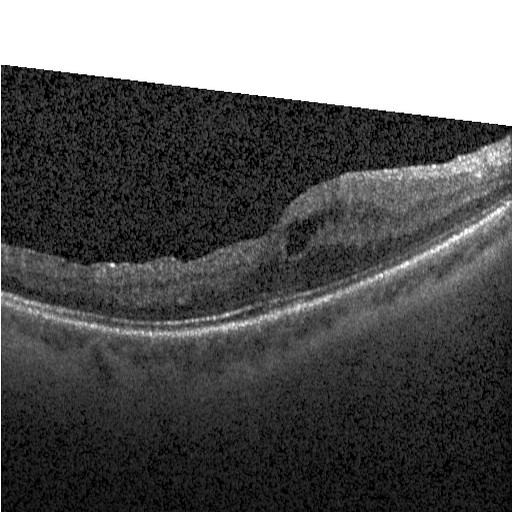
Optical coherence tomography B-scan. Acquired on a Heidelberg Spectralis. Fovea-centered. Spectral-domain OCT
The scan shows DME.